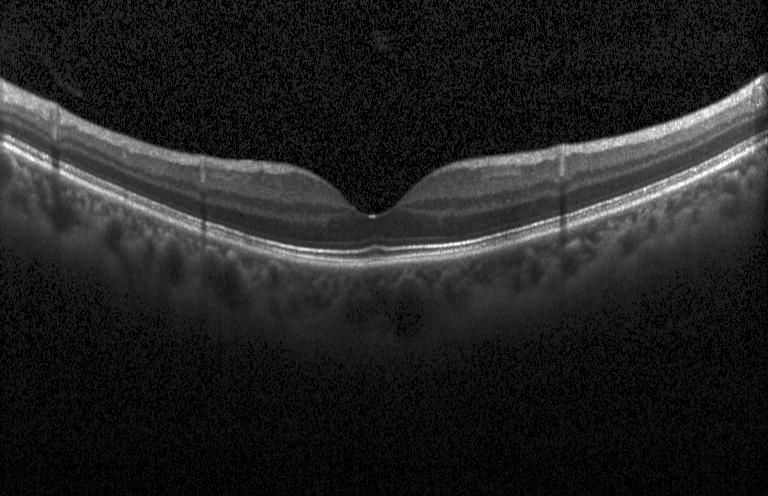 Finding: no CNV, DME, or drusen.